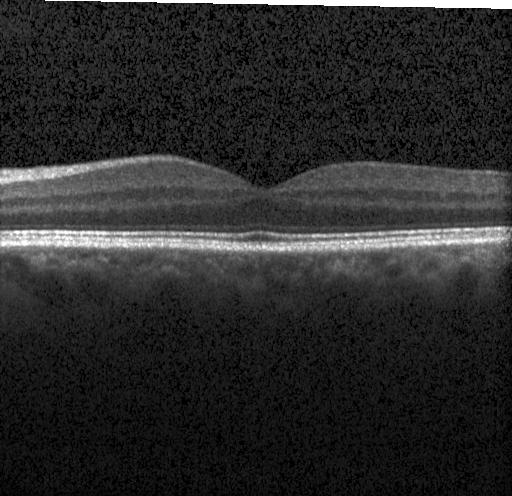
Optical coherence tomography B-scan — OCT finding: no choroidal neovascularization, no diabetic macular edema, and no drusen.